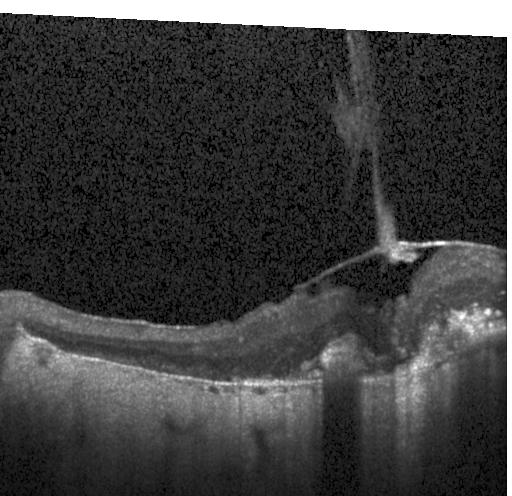

Through the macula; SD-OCT; retinal OCT B-scan; Heidelberg Spectralis OCT system
This B-scan demonstrates a choroidal neovascular membrane.